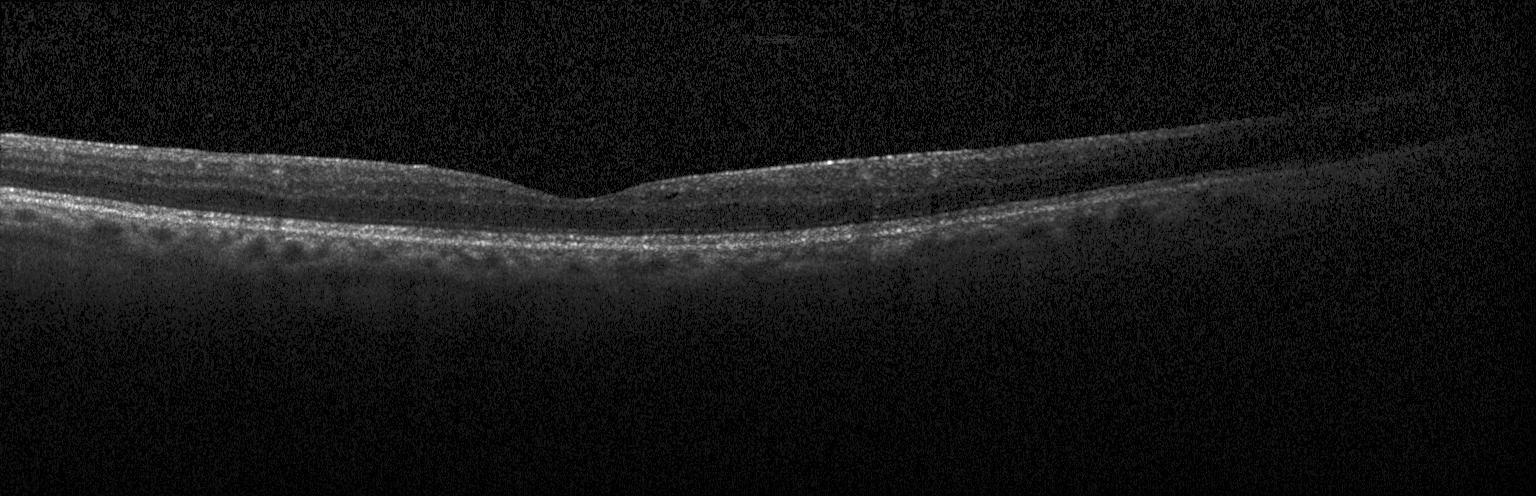
Retinal OCT cross-section; acquired on a Heidelberg Spectralis; macular scan; spectral-domain OCT.
Impression: no choroidal neovascularization, no diabetic macular edema, and no drusen.